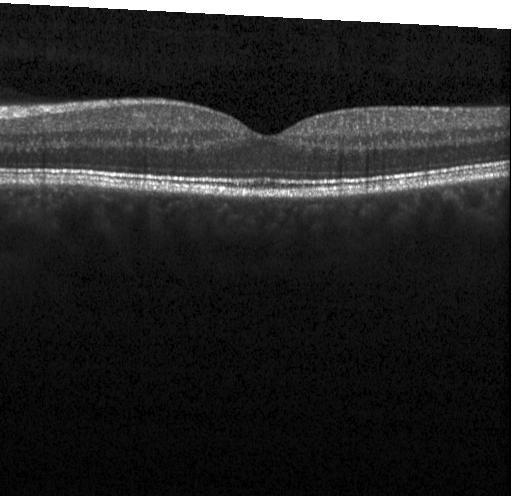

Spectral-domain OCT B-scan: no choroidal neovascularization, diabetic macular edema, or drusen.